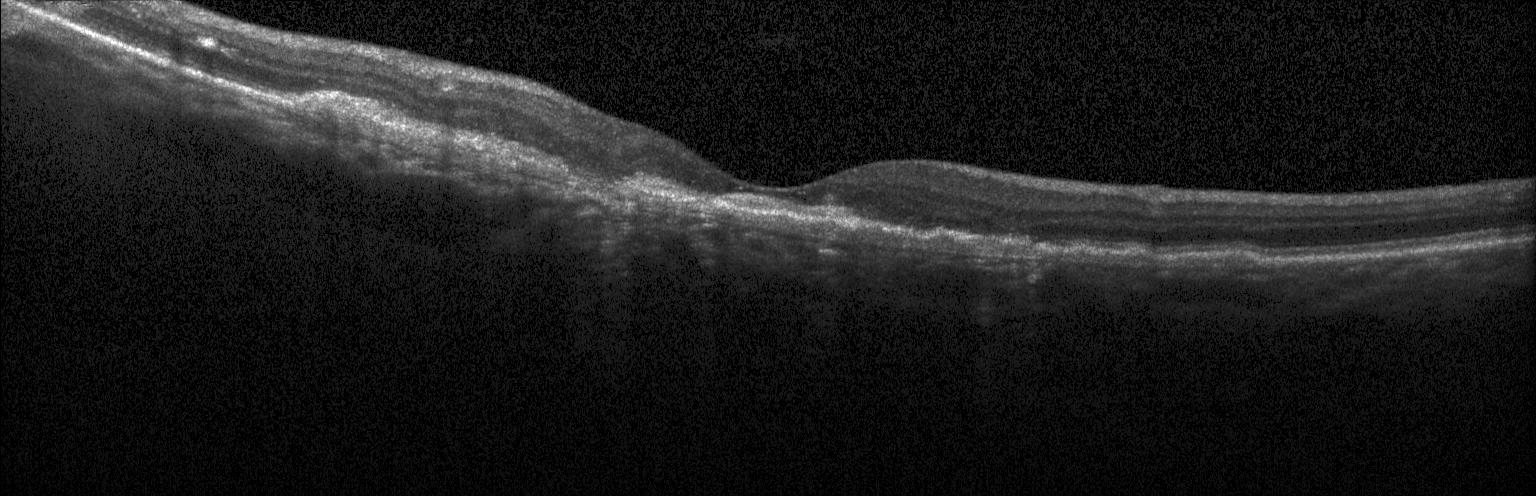
Optical coherence tomography scan
Choroidal neovascularization.